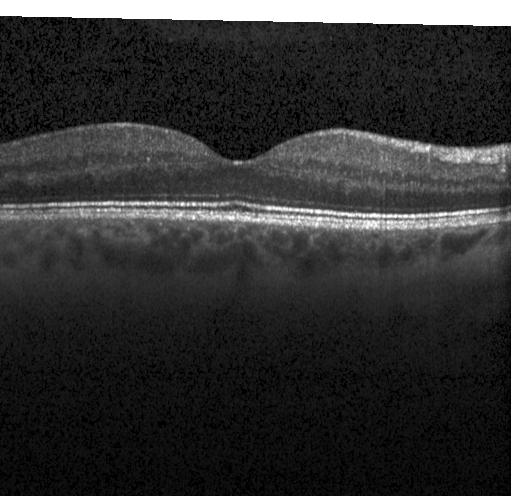
OCT B-scan · through the macula — OCT finding: no CNV, no DME, and no drusen.